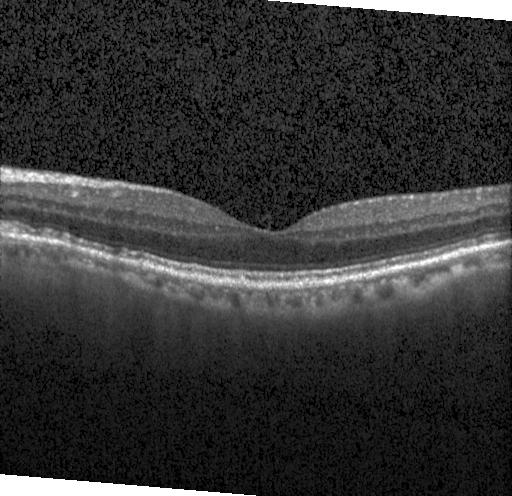 Spectral-domain OCT. OCT B-scan
Finding: no choroidal neovascularization, diabetic macular edema, or drusen.